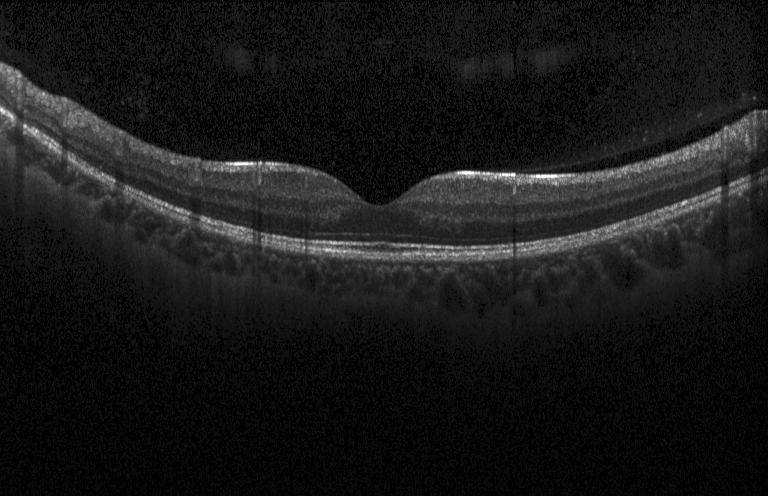

Finding: no CNV, DME, or drusen.